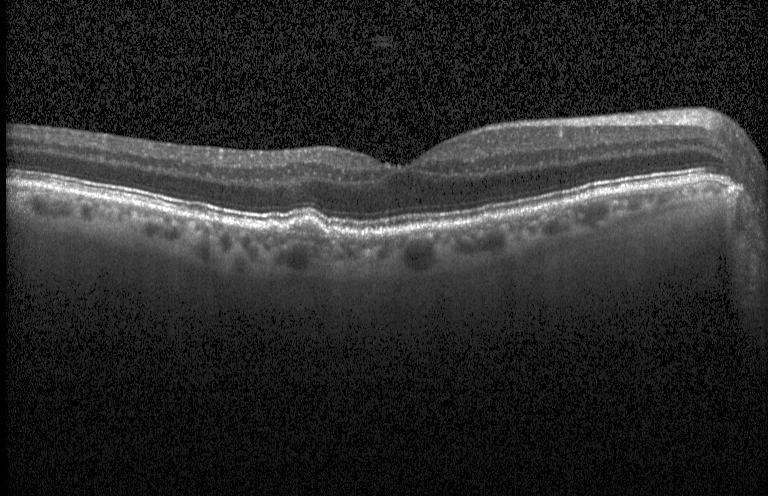

Retinal OCT cross-section. SD-OCT. Acquired on a Heidelberg Spectralis. Through the macula
Assessment: drusen.